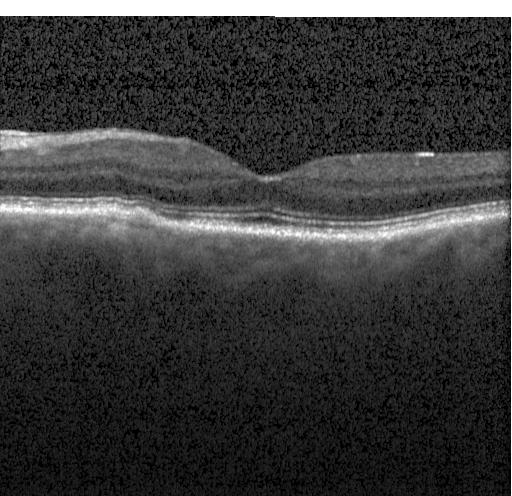

Fovea-centered, retinal OCT B-scan, instrument: Heidelberg Spectralis, SD-OCT — Diagnosis: sub-RPE drusenoid deposits.